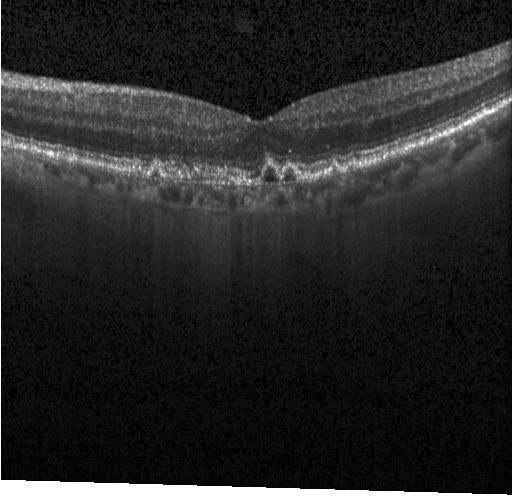

OCT B-scan; SD-OCT — Impression: a choroidal neovascular membrane.